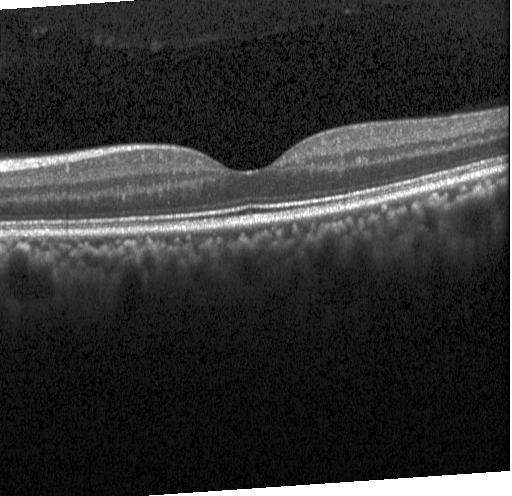

OCT B-scan showing neither choroidal neovascularization, diabetic macular edema, nor drusen.